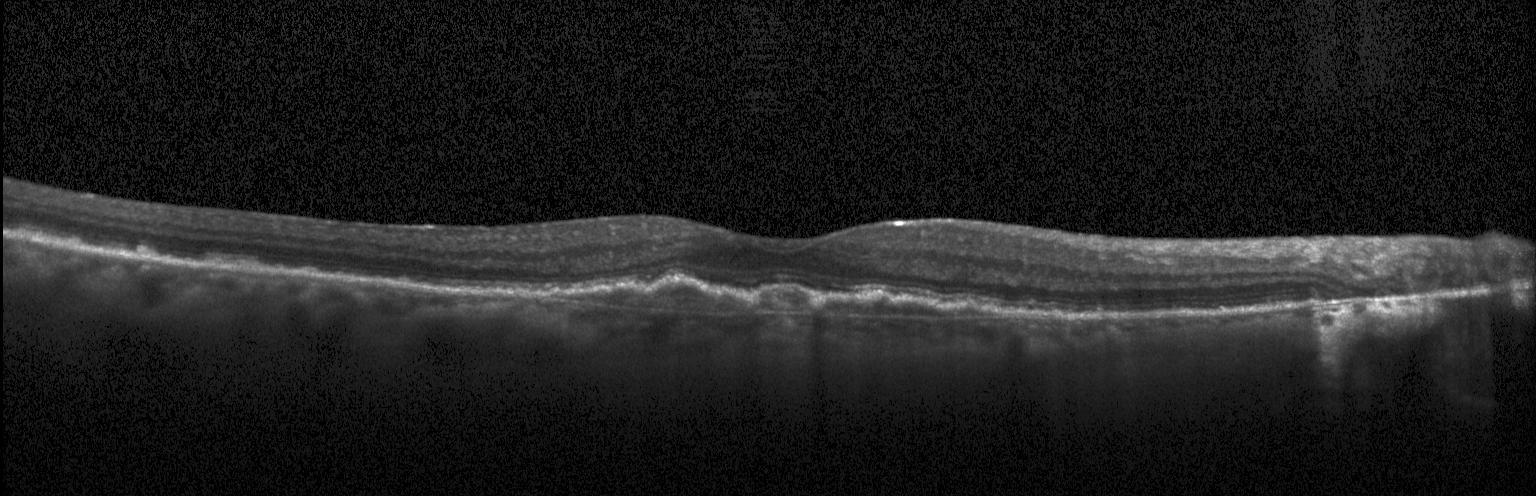
Retinal OCT B-scan.
Impression: choroidal neovascularization (CNV).